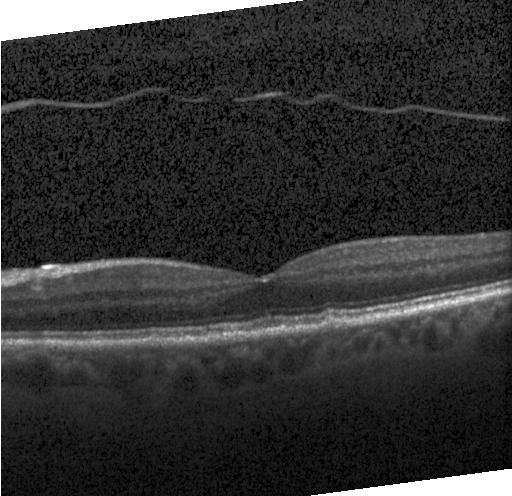
OCT line scan. Centered on the fovea. Instrument: Heidelberg Spectralis
The scan shows sub-RPE drusenoid deposits.